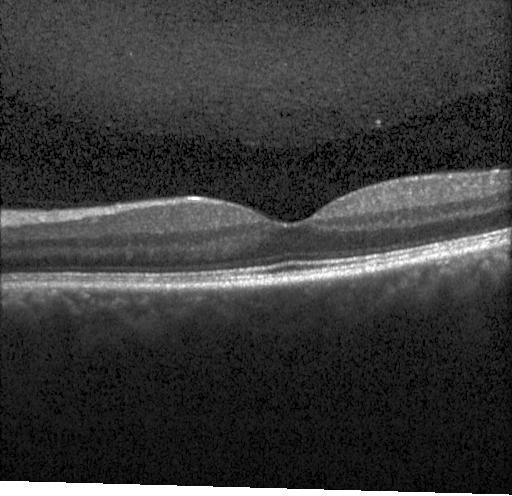

Spectral-domain OCT · OCT B-scan · through the macula — Finding: no evidence of CNV, DME, or drusen.